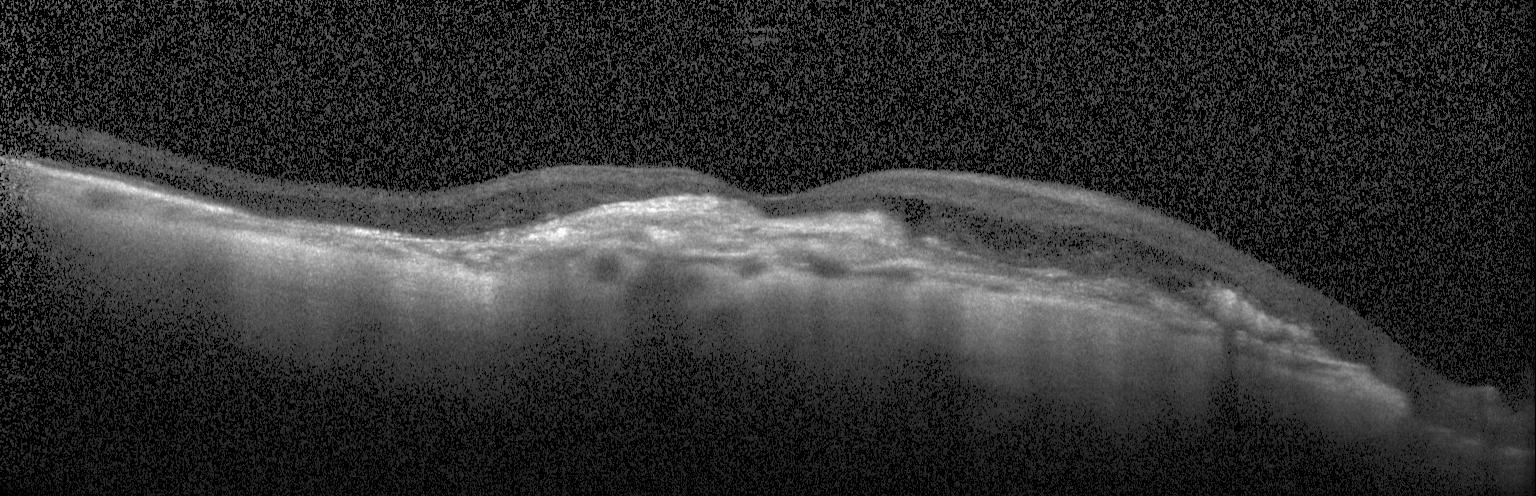
The scan shows CNV.